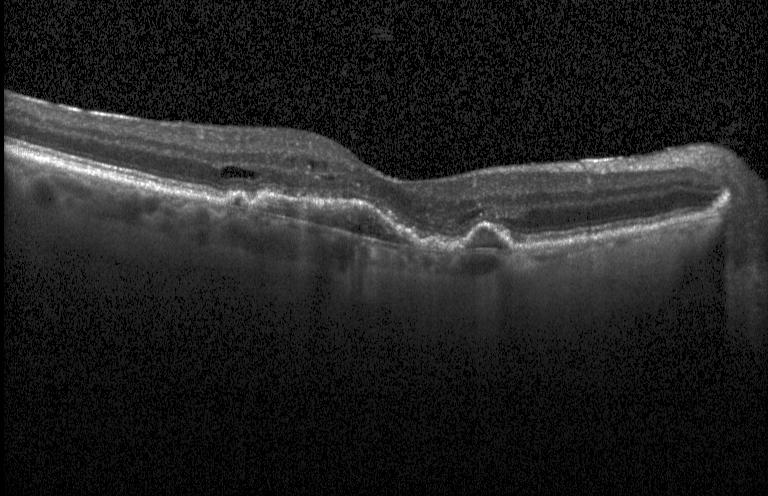 Diagnosis: a choroidal neovascular membrane.